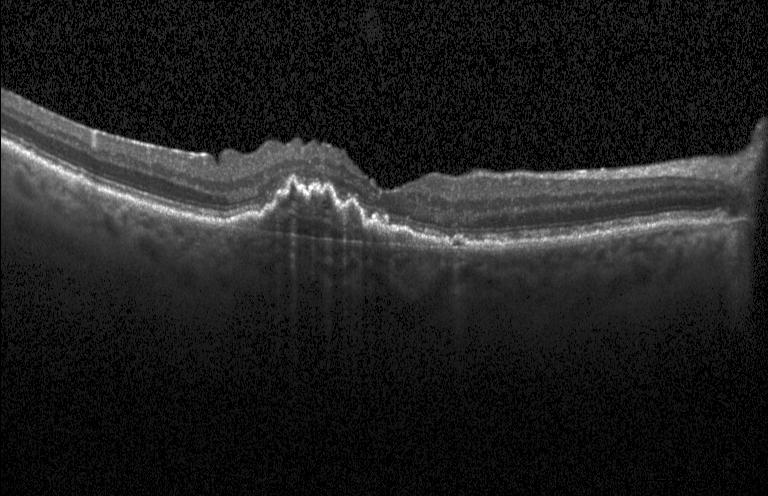 Instrument: Heidelberg Spectralis, optical coherence tomography B-scan
Finding: choroidal neovascularization (CNV).